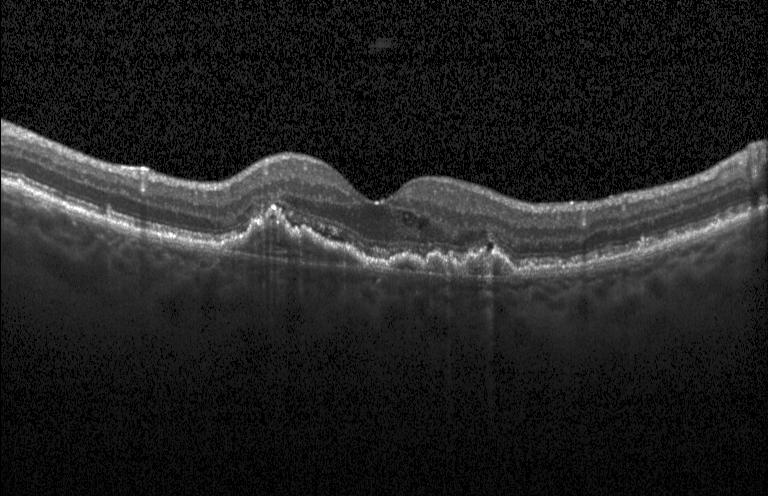 Horizontal scan through the fovea. OCT line scan
Diagnosis: a choroidal neovascular membrane.